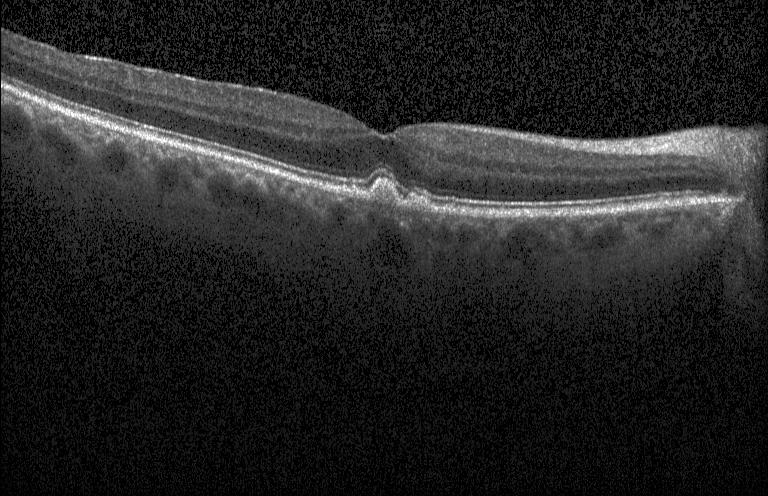 Impression: sub-RPE drusenoid deposits.